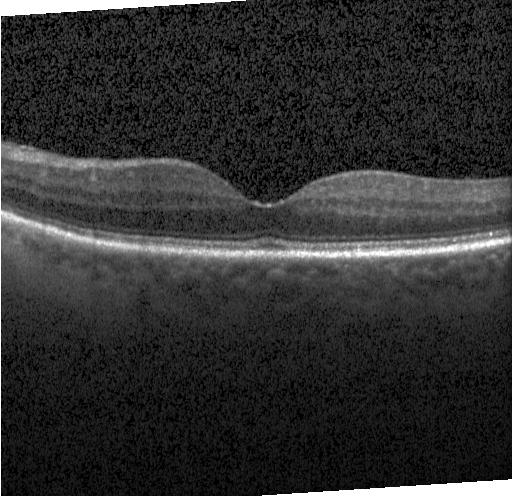

Heidelberg Spectralis OCT system; OCT line scan. This B-scan demonstrates no evidence of choroidal neovascularization, diabetic macular edema, or drusen.